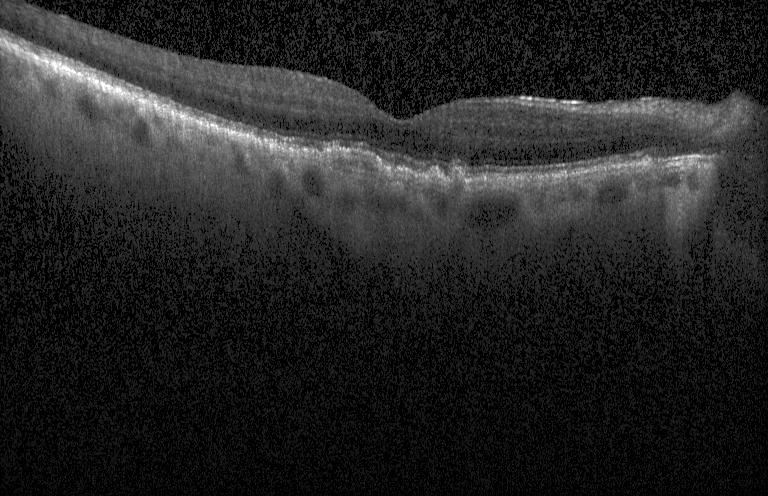
Retinal OCT B-scan. CNV.